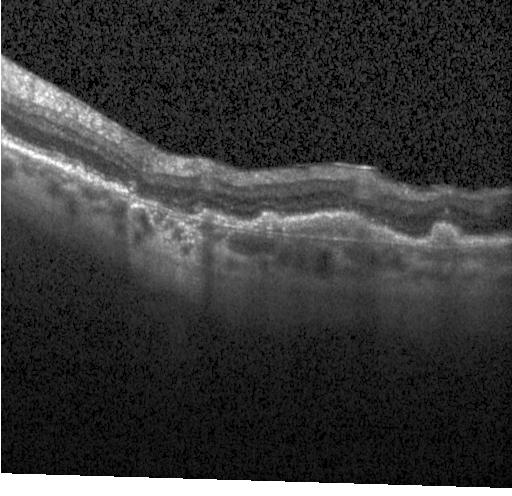 Spectral-domain optical coherence tomography · OCT B-scan.
Finding: choroidal neovascularization (CNV).